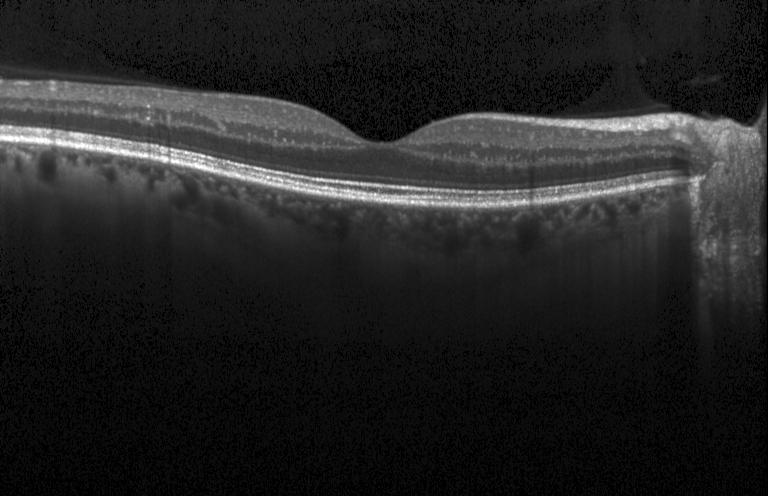 Impression: no choroidal neovascularization, diabetic macular edema, or drusen.